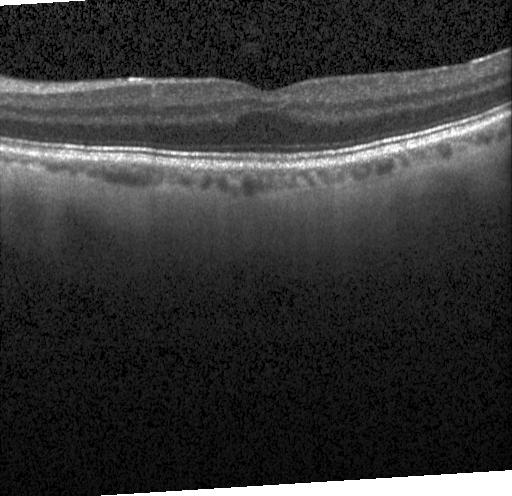

OCT B-scan. SD-OCT. Fovea-centered. Acquired on a Heidelberg Spectralis.
Finding: no choroidal neovascularization, no diabetic macular edema, and no drusen.